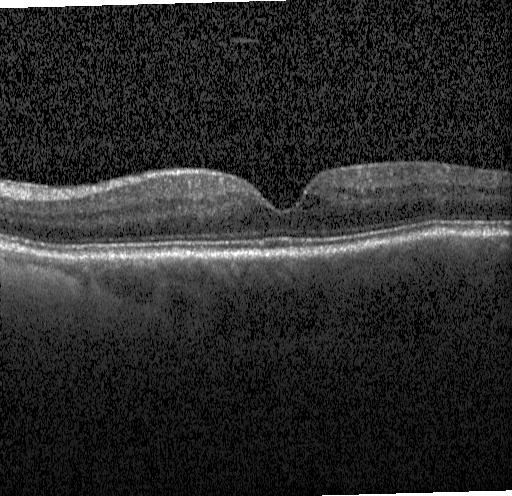
Impression: DME.